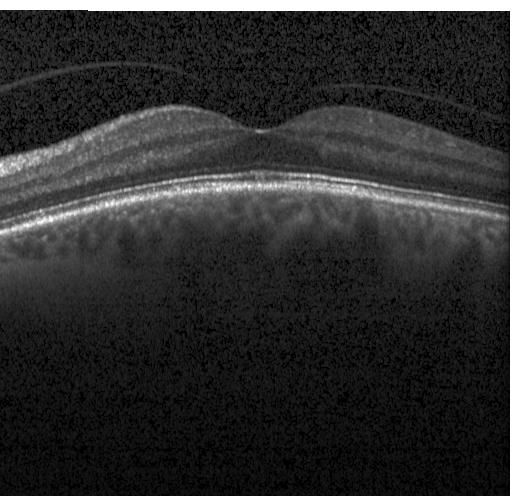 Macular OCT: neither choroidal neovascularization, diabetic macular edema, nor drusen.